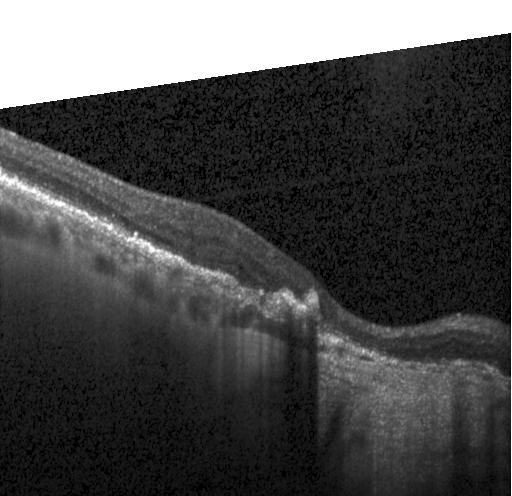
OCT B-scan
Finding: CNV.